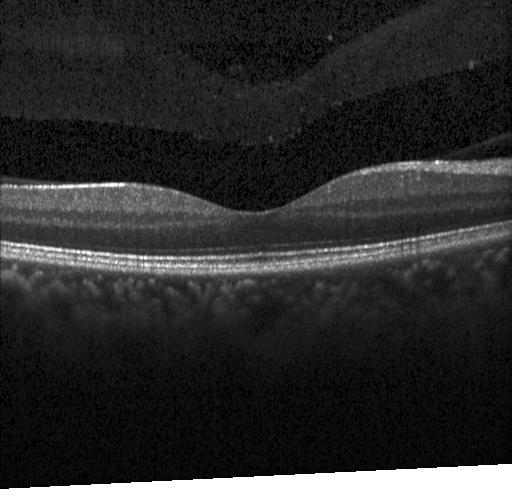 OCT B-scan. The scan shows no choroidal neovascularization, no diabetic macular edema, and no drusen.